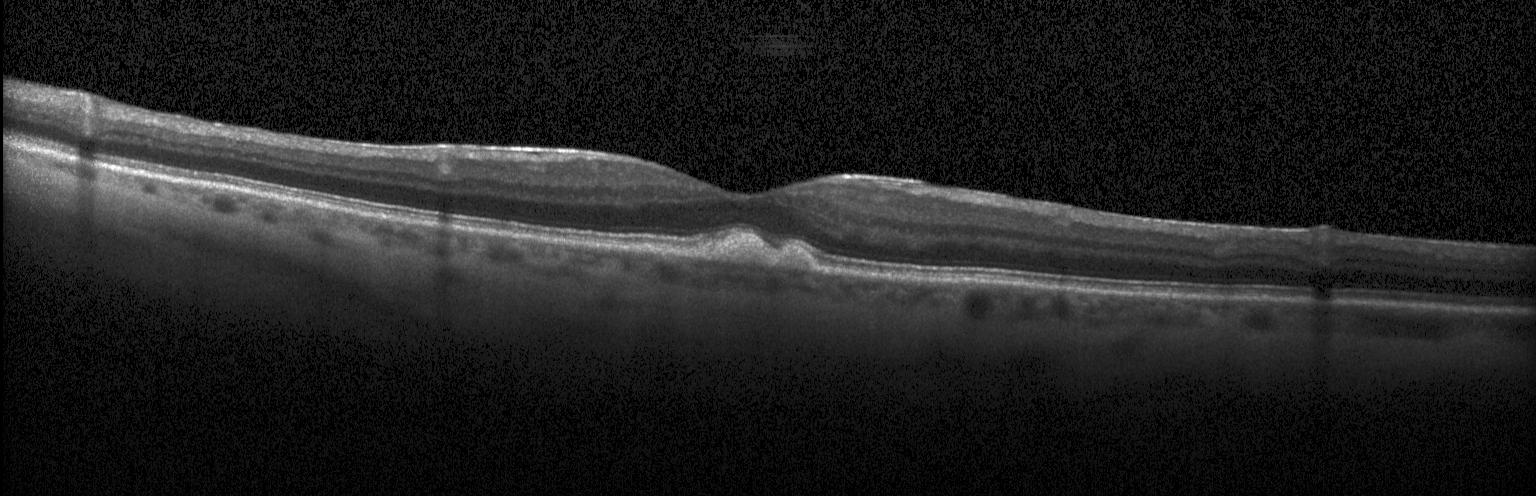

OCT B-scan, SD-OCT. Impression: drusen.